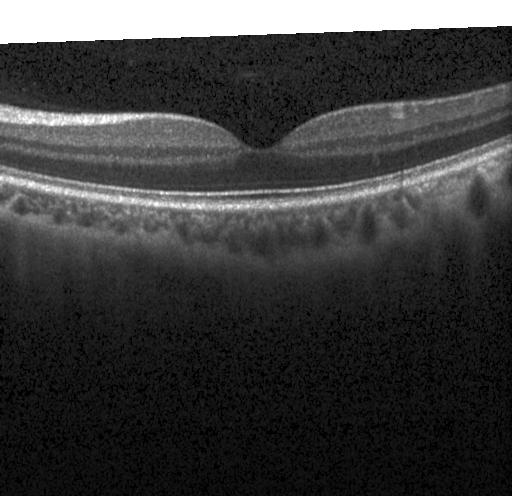
Centered on the fovea. OCT B-scan. Assessment: no evidence of choroidal neovascularization, diabetic macular edema, or drusen.